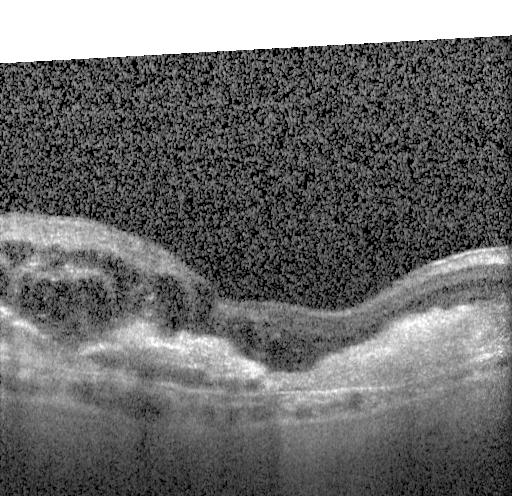 Diagnosis: a choroidal neovascular membrane.